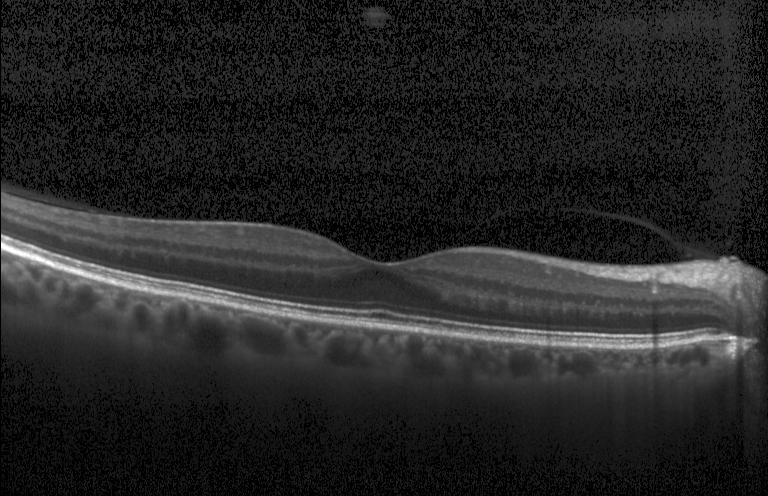

OCT line scan. Macular scan. SD-OCT. Heidelberg Spectralis OCT system. Diagnosis: no choroidal neovascularization, no diabetic macular edema, and no drusen.